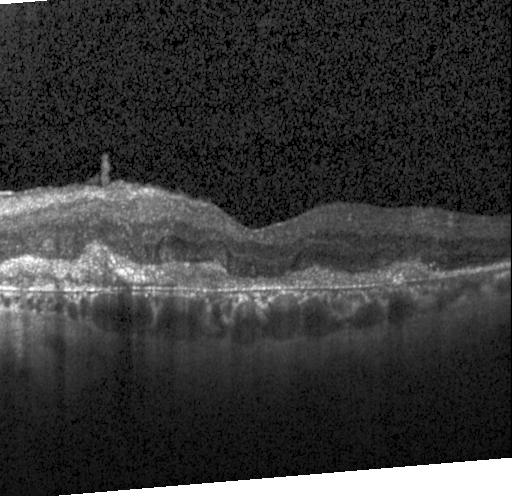 Macular OCT: a choroidal neovascular membrane.